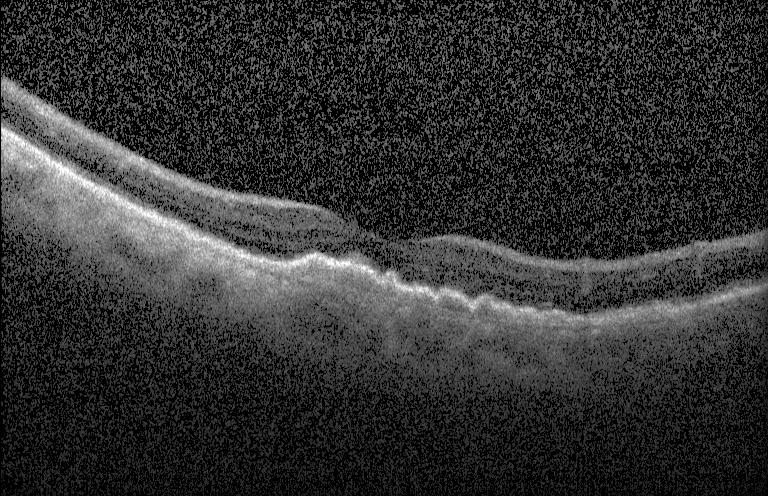

Retinal OCT B-scan; acquired on a Heidelberg Spectralis — Choroidal neovascularization.